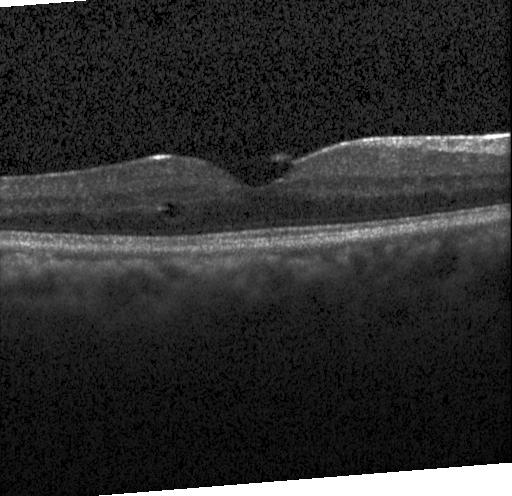

Optical coherence tomography scan
OCT finding: diabetic macular edema (DME).